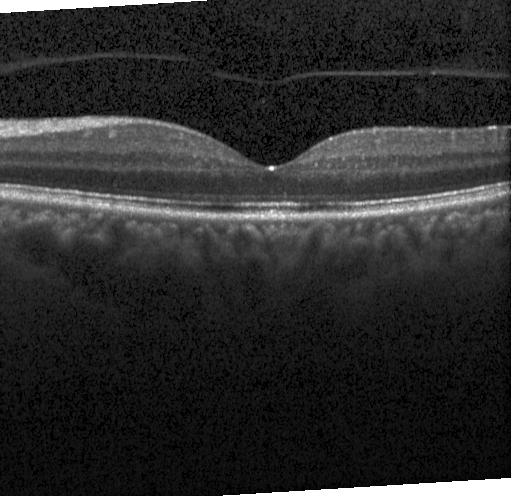 Impression: no evidence of CNV, DME, or drusen.